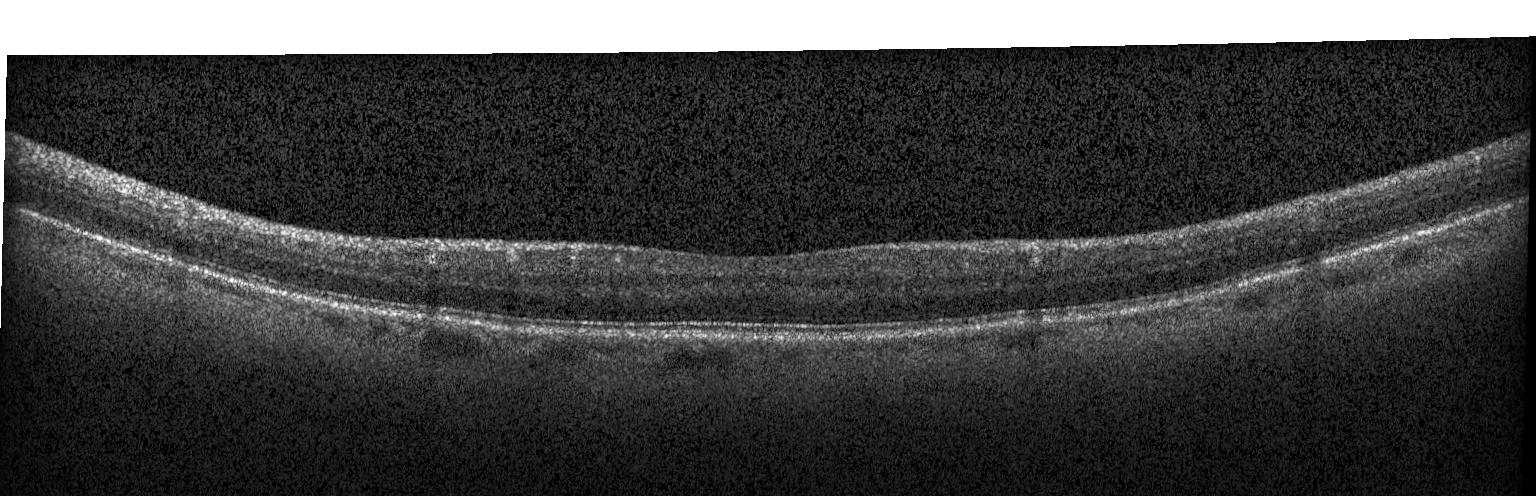 OCT scan showing neither CNV, DME, nor drusen.